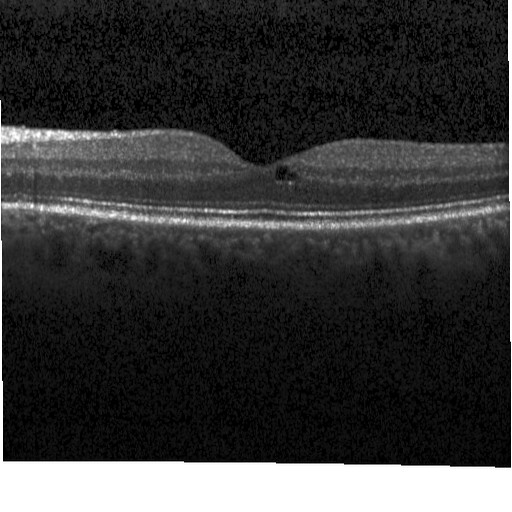
OCT finding: DME.